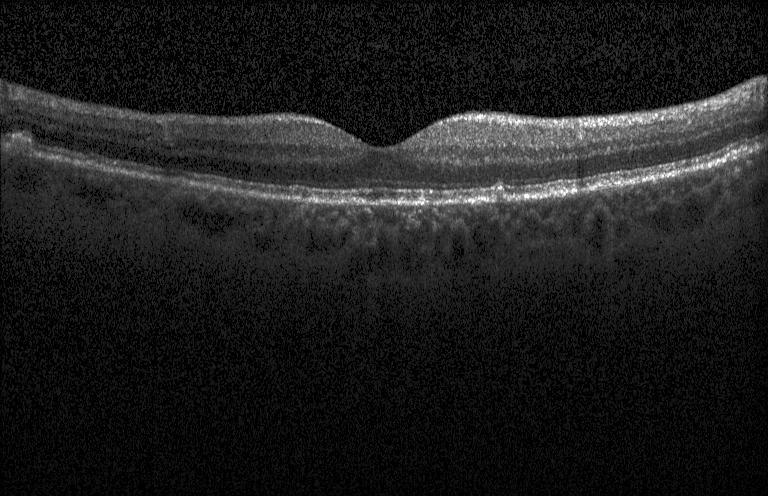 Horizontal scan through the fovea, Heidelberg Spectralis OCT system, retinal OCT cross-section, spectral-domain OCT. Impression: sub-RPE drusenoid deposits.